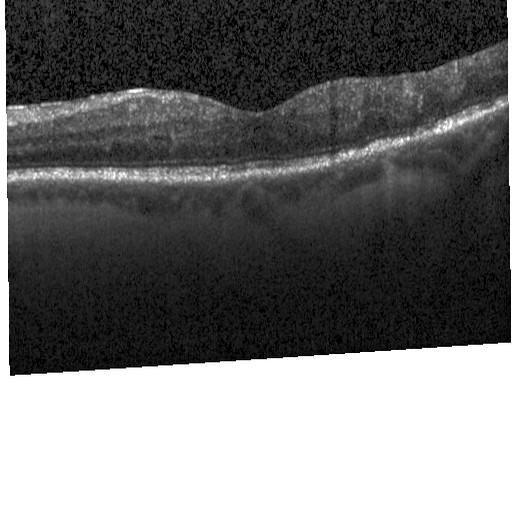

Horizontal scan through the fovea, spectral-domain optical coherence tomography, Heidelberg Spectralis OCT system, OCT B-scan. Diabetic macular edema (DME).